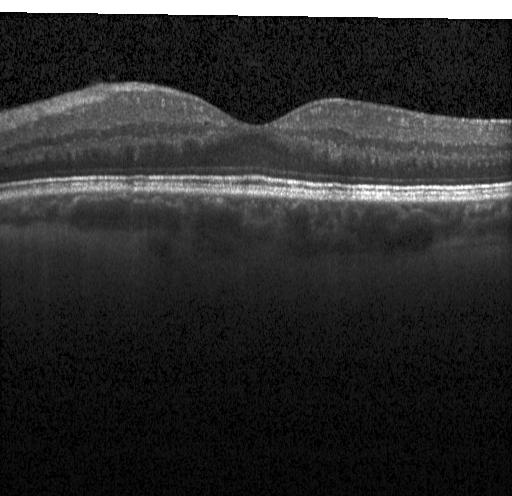
OCT scan showing no choroidal neovascularization, diabetic macular edema, or drusen.